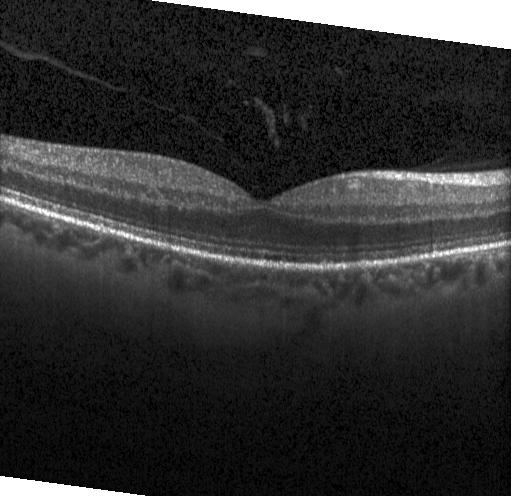
Macular scan; optical coherence tomography scan; spectral-domain OCT; Heidelberg Spectralis OCT system
The scan shows no evidence of choroidal neovascularization, diabetic macular edema, or drusen.